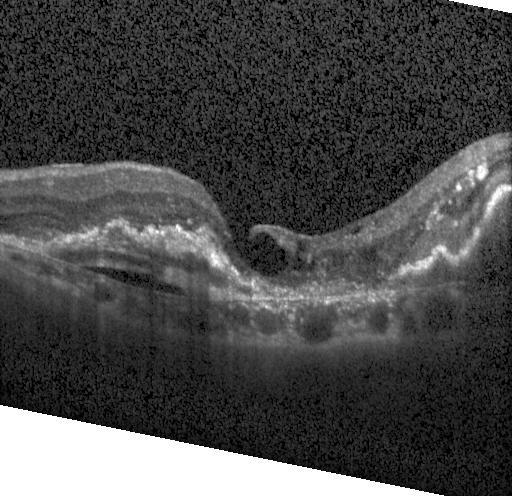
Optical coherence tomography scan, horizontal scan through the fovea
This B-scan demonstrates a choroidal neovascular membrane.